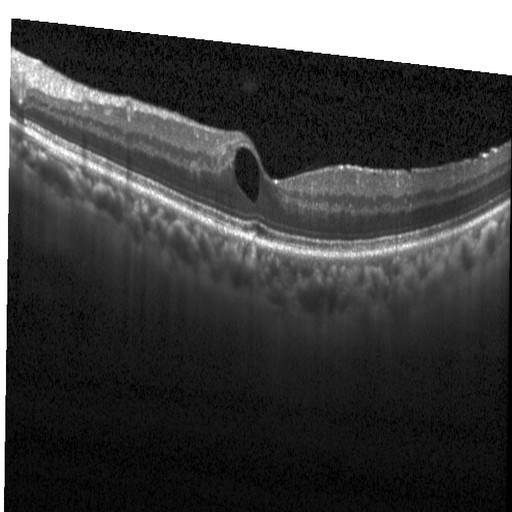 Optical coherence tomography B-scan. Dx: diabetic macular edema (DME).